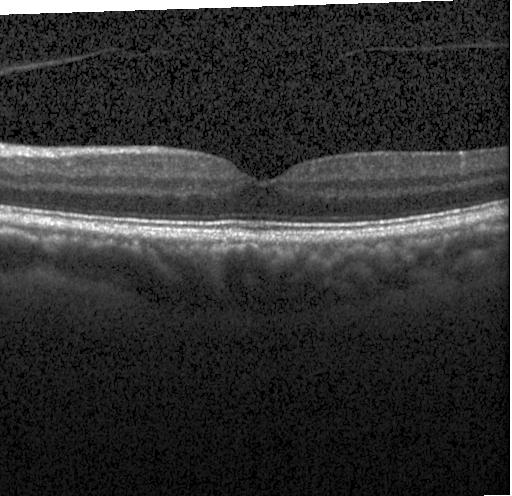
Macular OCT: neither choroidal neovascularization, diabetic macular edema, nor drusen.